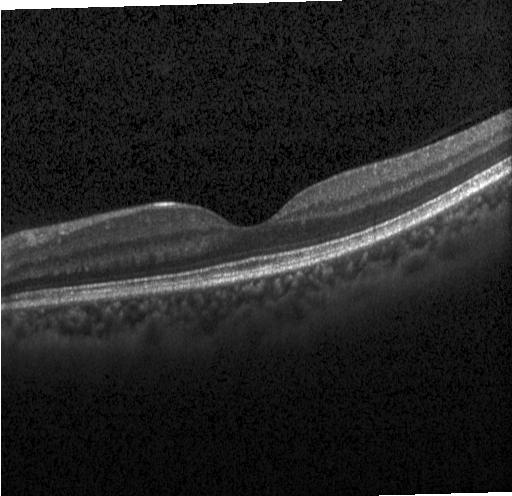
Optical coherence tomography B-scan.
Impression: no choroidal neovascularization, no diabetic macular edema, and no drusen.